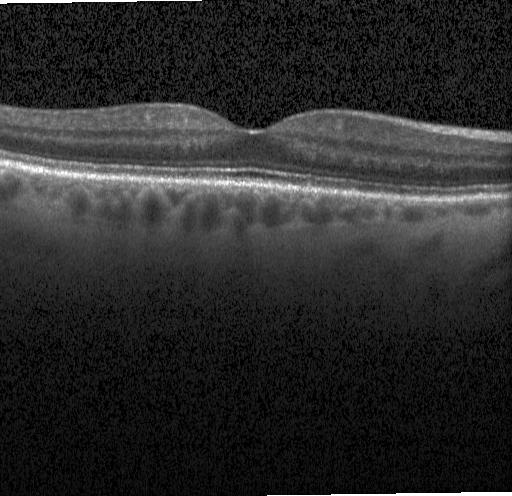
Spectral-domain optical coherence tomography. Optical coherence tomography B-scan. Instrument: Heidelberg Spectralis. Through the macula.
Assessment: no CNV, DME, or drusen.